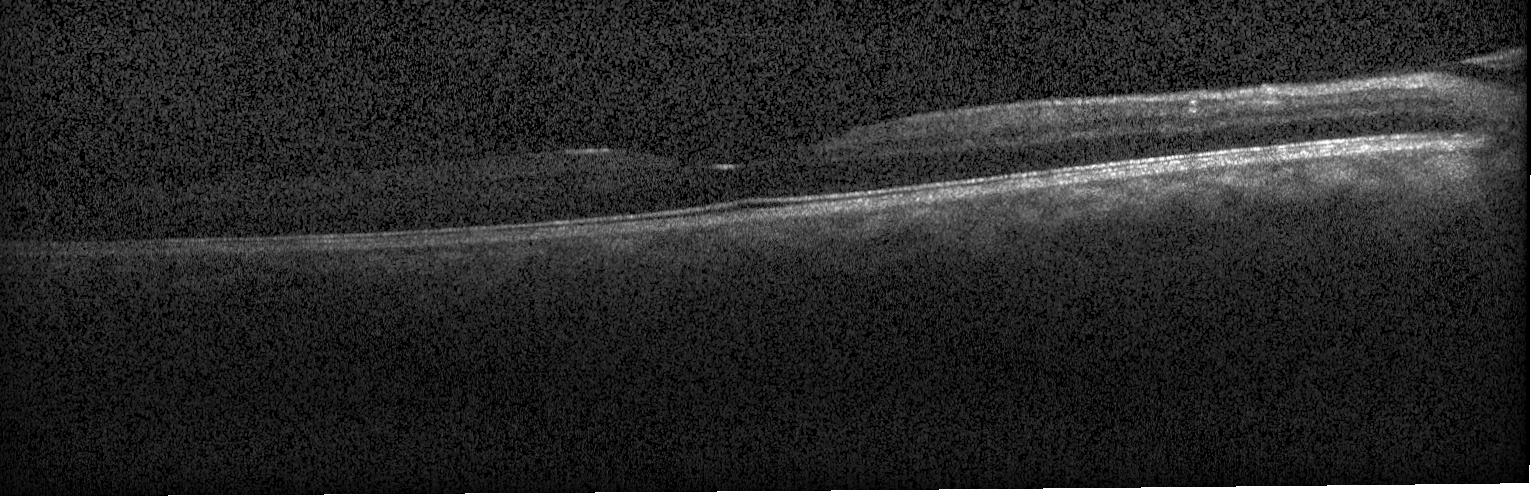
OCT finding: no choroidal neovascularization, diabetic macular edema, or drusen.